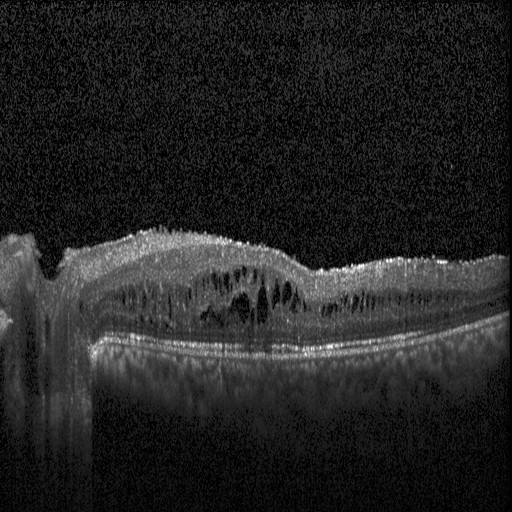

SD-OCT · retinal OCT B-scan — The scan shows diabetic macular edema (DME).